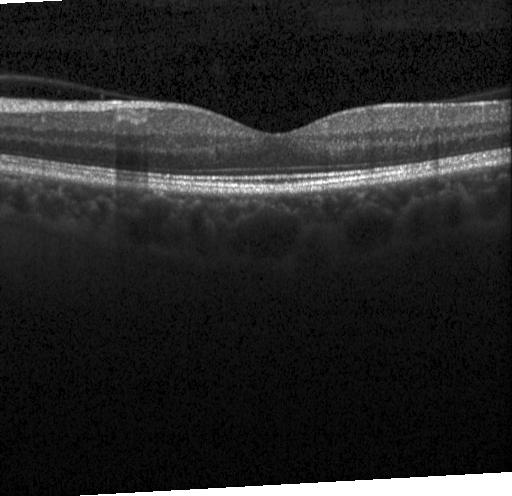
Spectral-domain optical coherence tomography · horizontal scan through the fovea · OCT line scan — The scan shows no choroidal neovascularization, no diabetic macular edema, and no drusen.